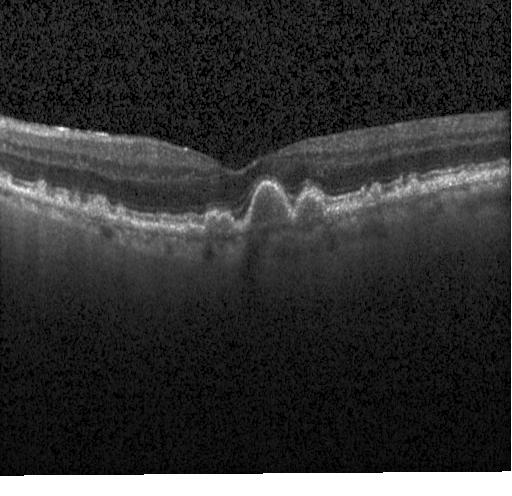 Horizontal scan through the fovea, OCT line scan — Impression: sub-RPE drusenoid deposits.